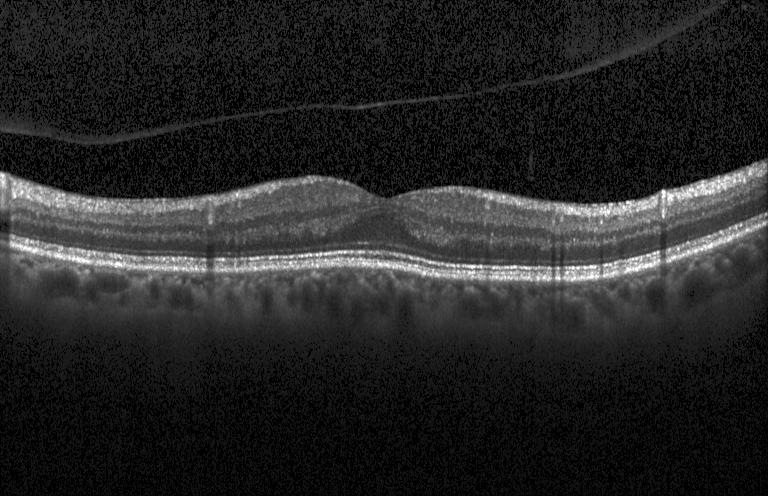 Spectral-domain OCT. OCT line scan. Heidelberg Spectralis OCT system — Assessment: no choroidal neovascularization, no diabetic macular edema, and no drusen.